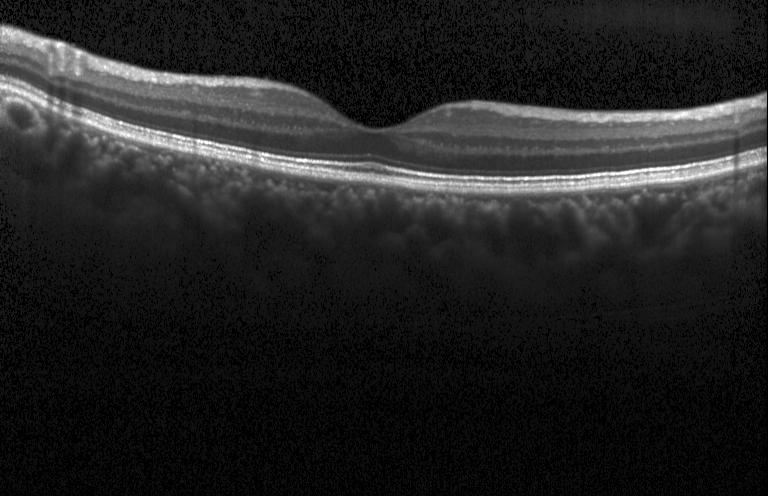

Through the macula; instrument: Heidelberg Spectralis; retinal OCT B-scan. No choroidal neovascularization, no diabetic macular edema, and no drusen.